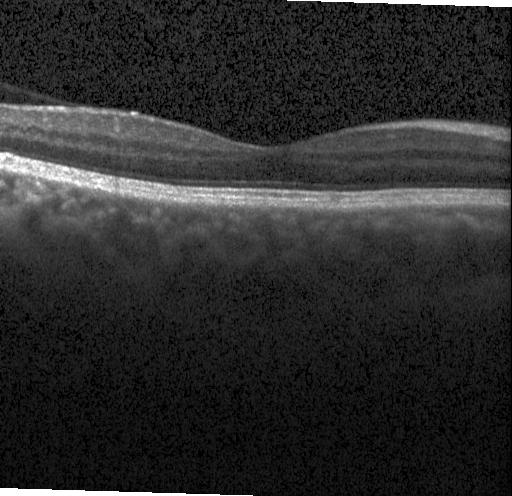
Retinal OCT cross-section. Dx: no evidence of CNV, DME, or drusen.